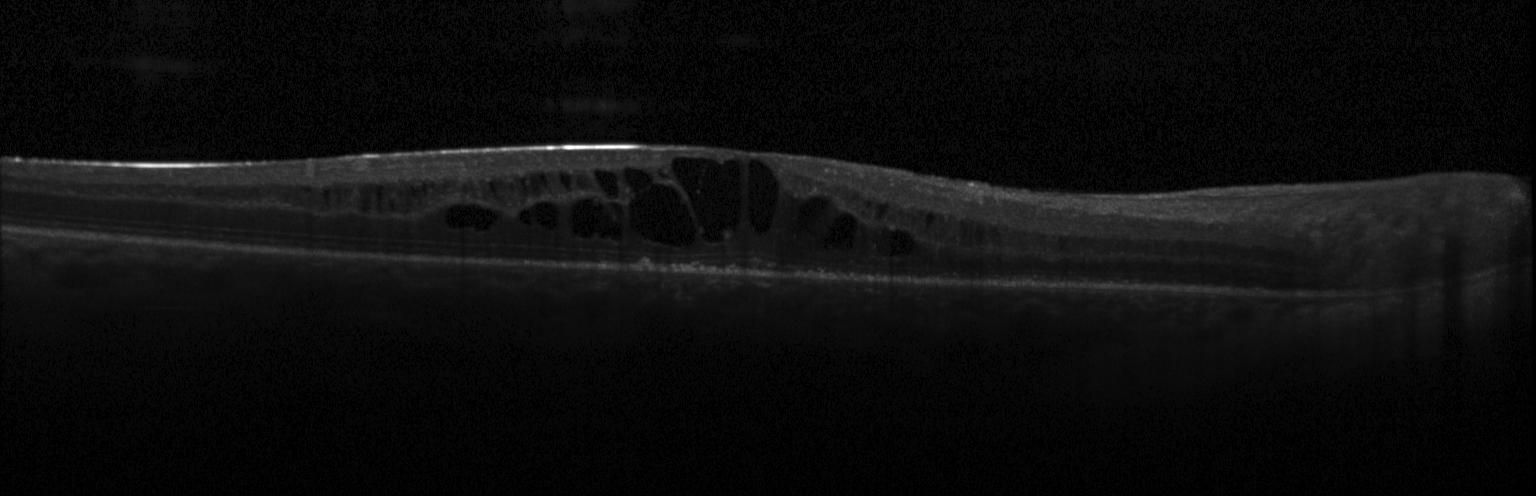

Acquired on a Heidelberg Spectralis, horizontal scan through the fovea, OCT line scan — Impression: diabetic macular edema (DME).